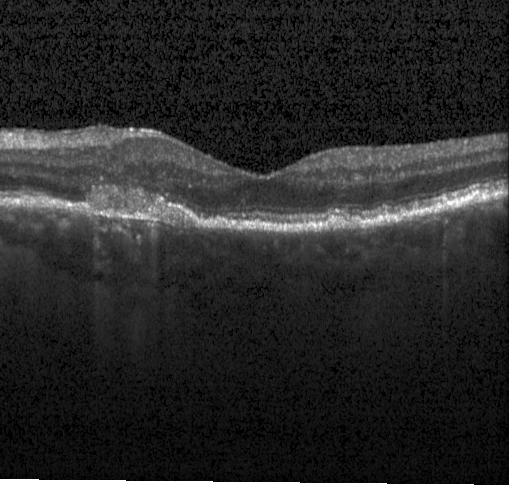
Diagnosis: choroidal neovascularization (CNV).